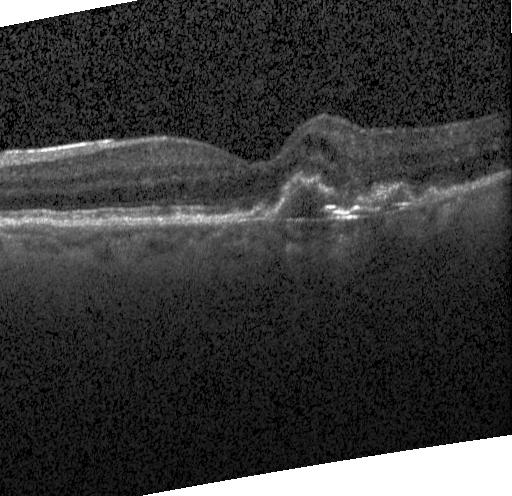
Macular scan, OCT line scan — This B-scan demonstrates CNV.